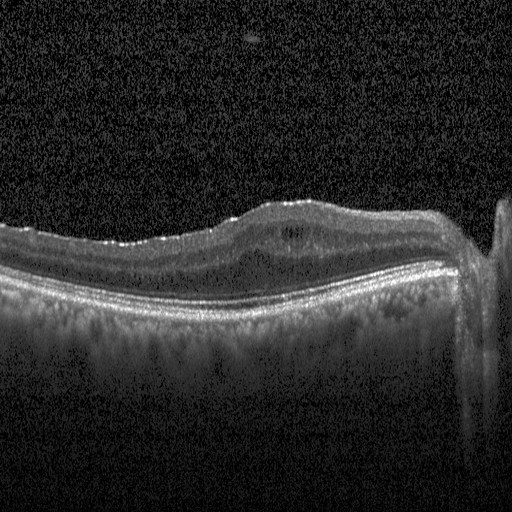

OCT B-scan; horizontal scan through the fovea; acquired on a Heidelberg Spectralis; spectral-domain optical coherence tomography.
The scan shows DME.